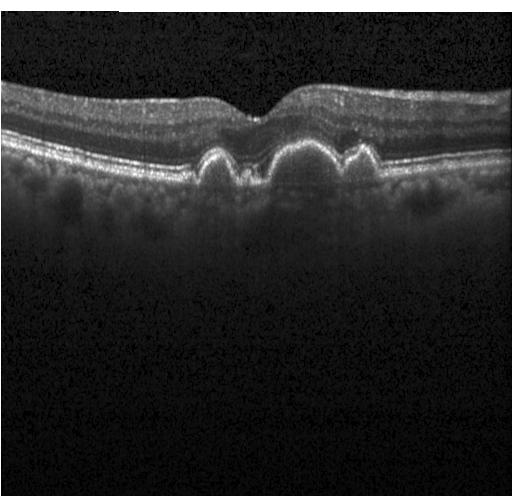 OCT finding: sub-RPE drusenoid deposits.